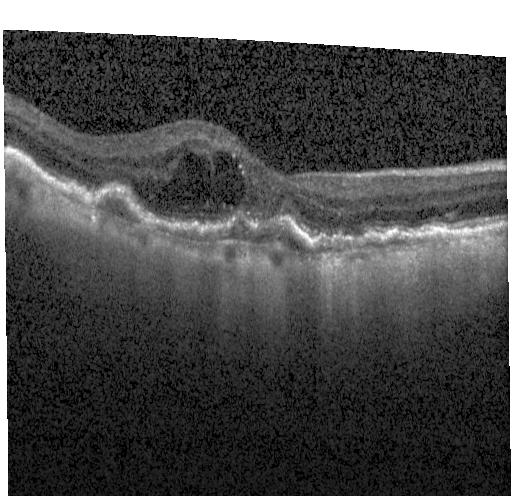

OCT line scan · spectral-domain OCT · through the macula · Heidelberg Spectralis — Finding: choroidal neovascularization (CNV).